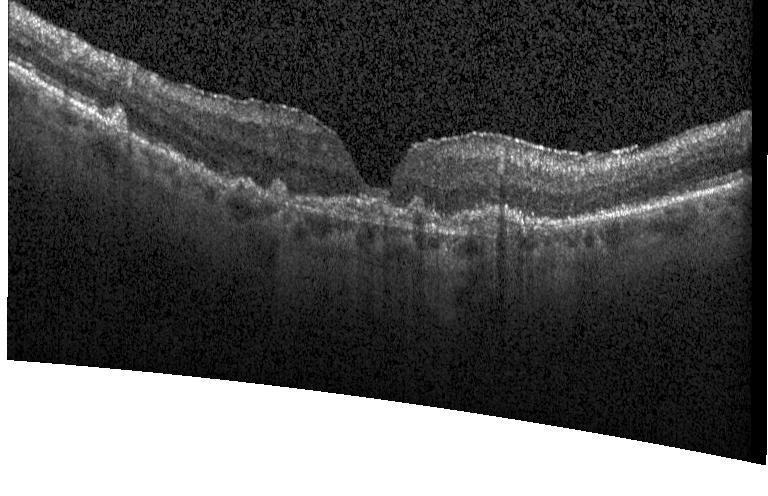
Diagnosis: choroidal neovascularization.